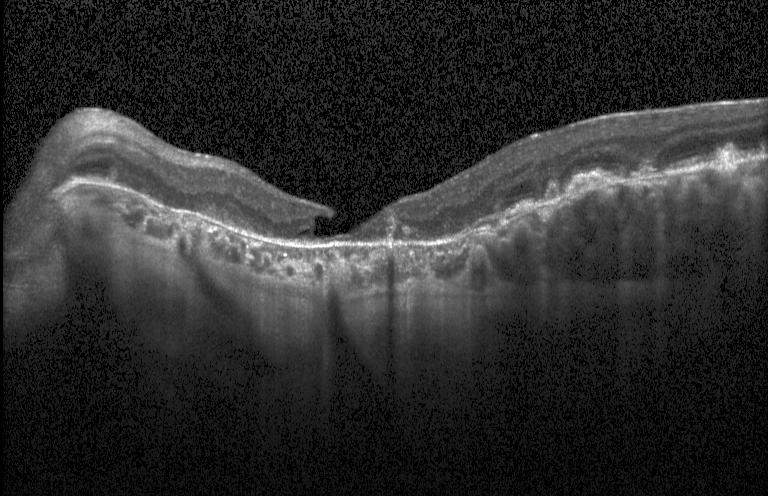 Impression: choroidal neovascularization (CNV).